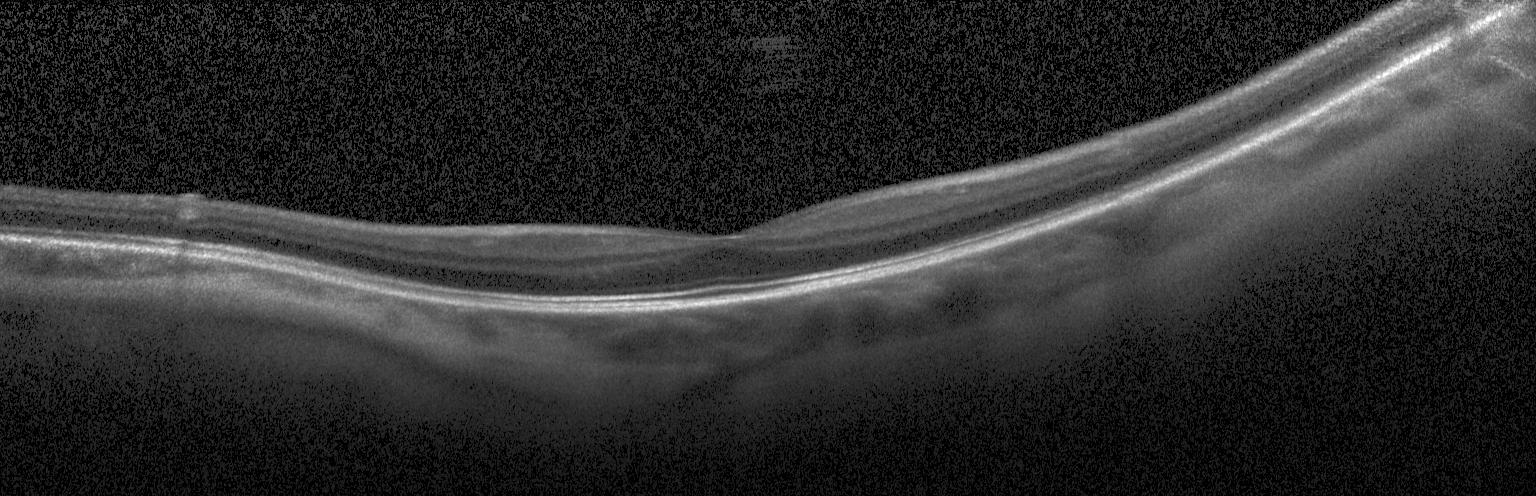 Diagnosis: no CNV, DME, or drusen.